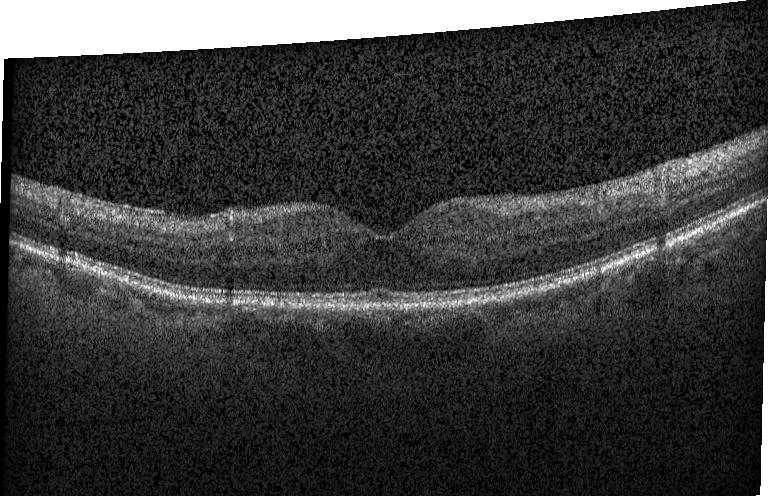
Retinal OCT cross-section. The scan shows neither choroidal neovascularization, diabetic macular edema, nor drusen.